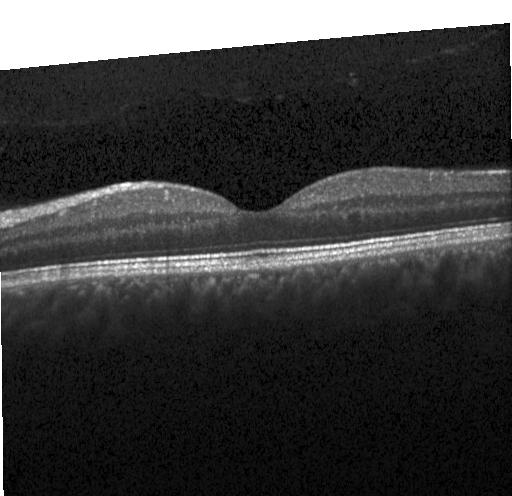
Spectral-domain OCT, optical coherence tomography scan
The scan shows no evidence of CNV, DME, or drusen.